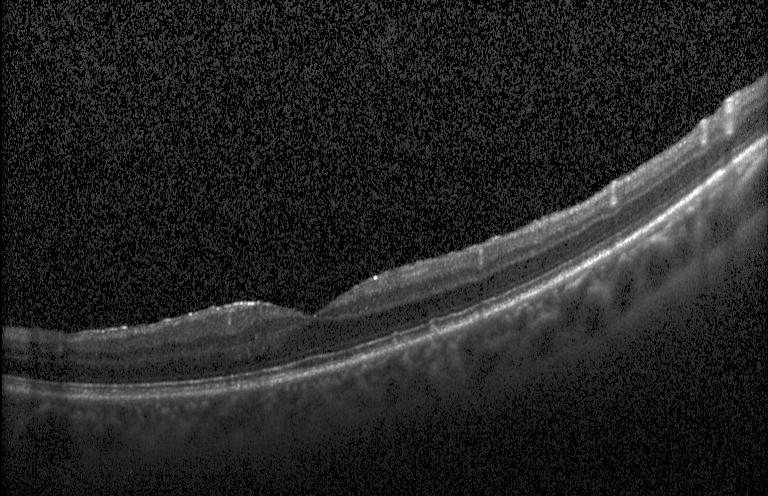
Diagnosis: drusen.